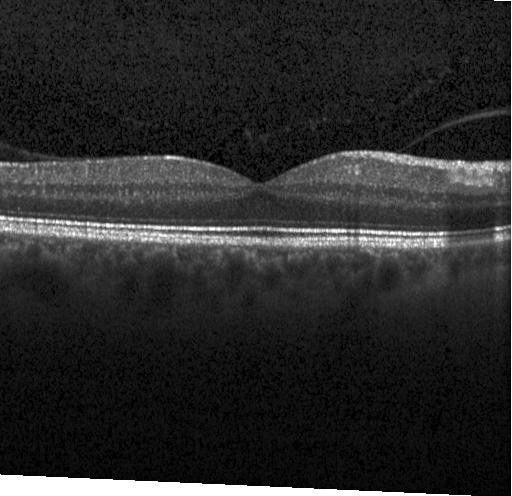
Impression: no evidence of choroidal neovascularization, diabetic macular edema, or drusen.